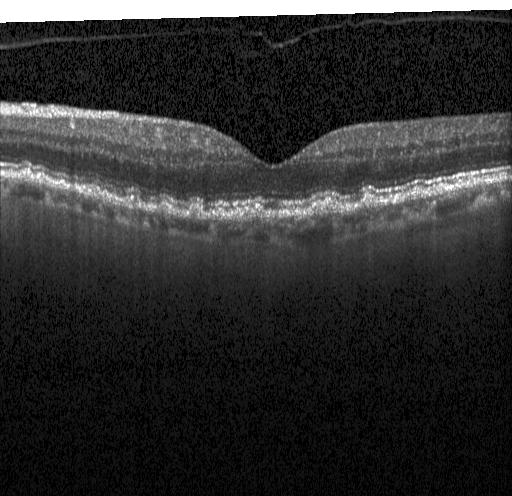
OCT B-scan.
This B-scan demonstrates sub-RPE drusenoid deposits.